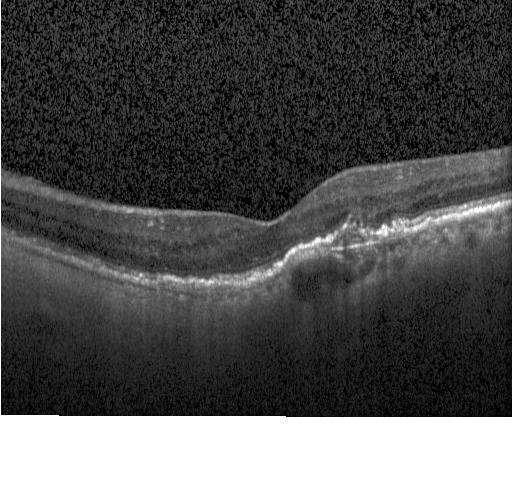
Assessment: a choroidal neovascular membrane.